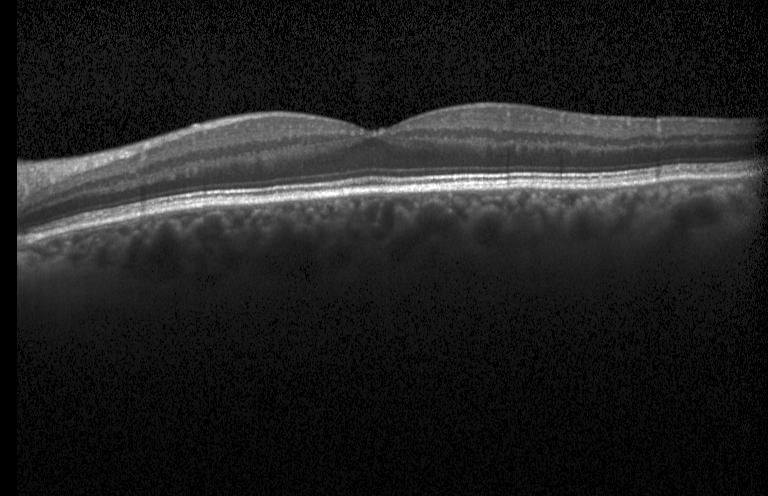
Assessment: no evidence of CNV, DME, or drusen.